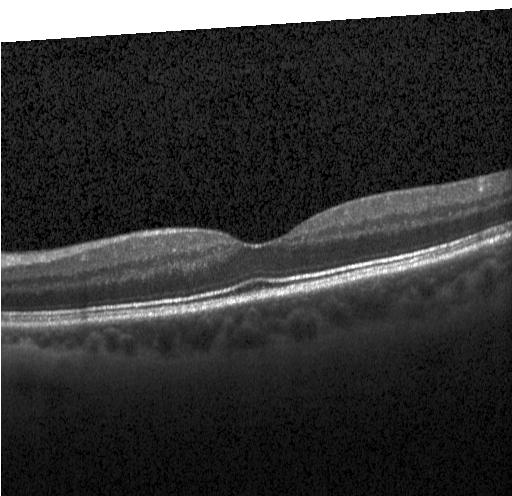
Finding: no choroidal neovascularization, no diabetic macular edema, and no drusen.